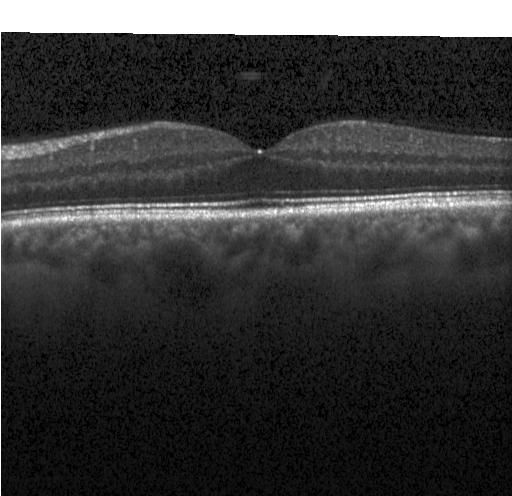
SD-OCT; Heidelberg Spectralis OCT system; retinal OCT B-scan; horizontal scan through the fovea. Dx: no choroidal neovascularization, no diabetic macular edema, and no drusen.